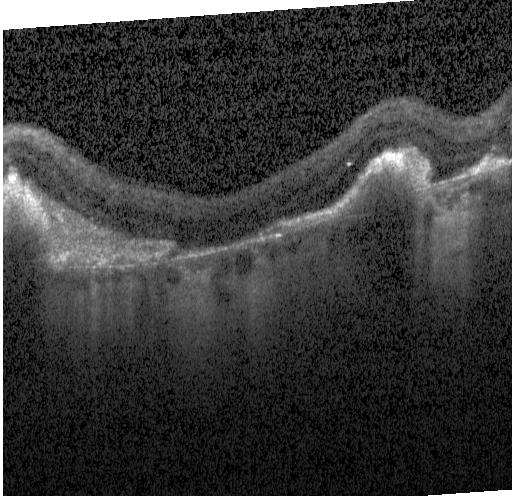
Macular OCT: a choroidal neovascular membrane.